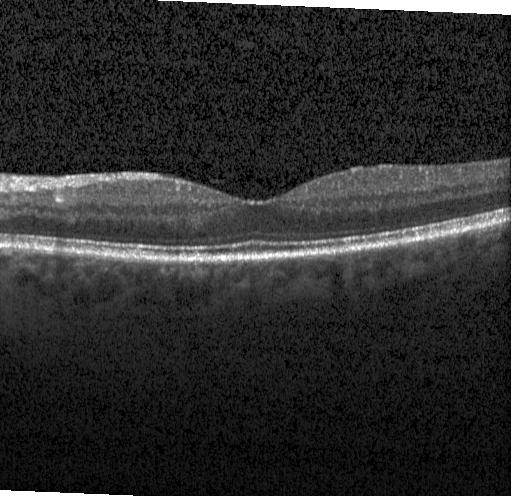 Retinal OCT cross-section showing no choroidal neovascularization, no diabetic macular edema, and no drusen.